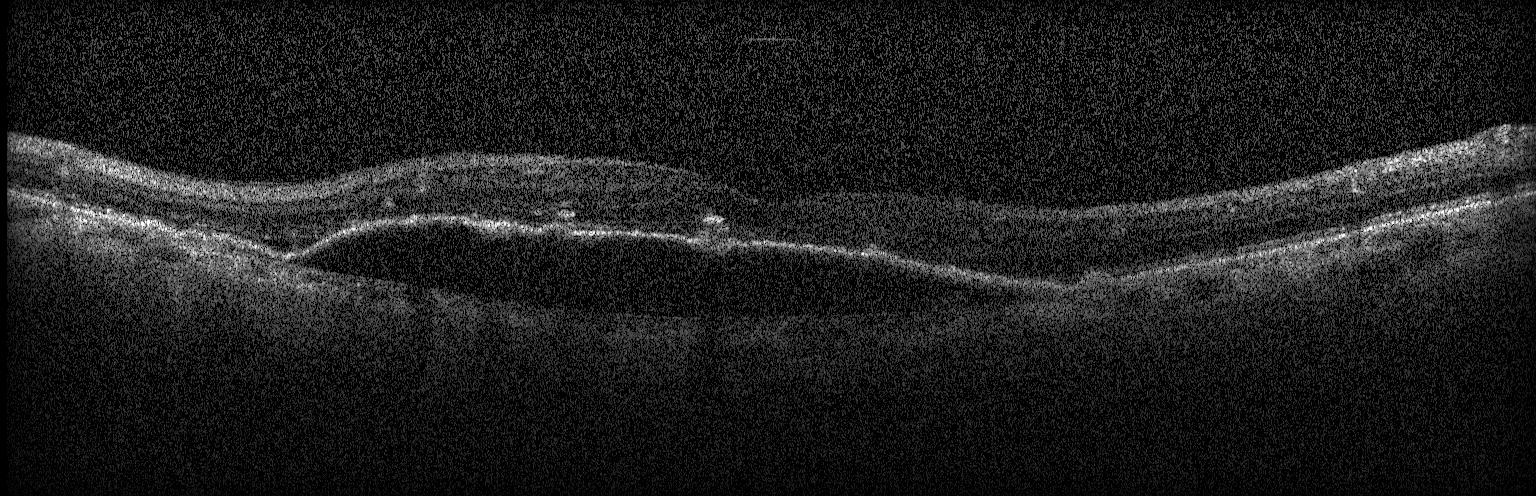 Spectral-domain OCT; retinal OCT cross-section; acquired on a Heidelberg Spectralis; macular scan
OCT finding: choroidal neovascularization (CNV).